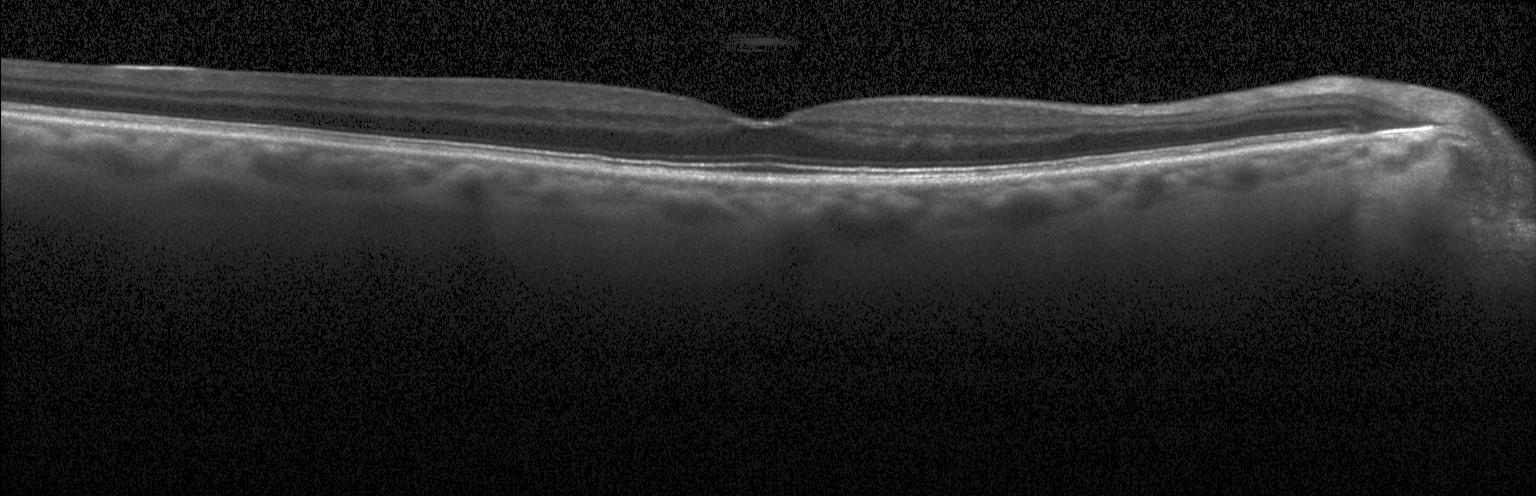
Optical coherence tomography scan — Impression: no choroidal neovascularization, no diabetic macular edema, and no drusen.